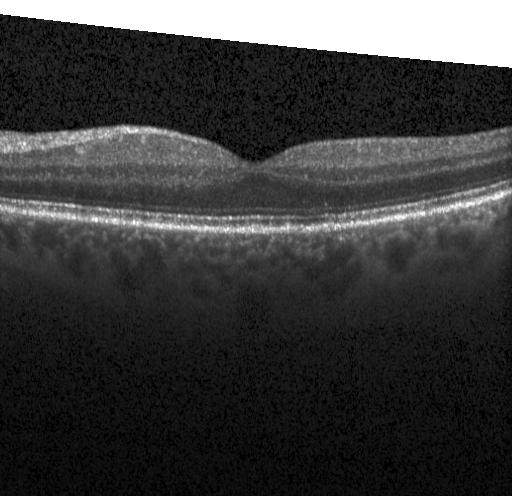 Finding: no choroidal neovascularization, diabetic macular edema, or drusen.